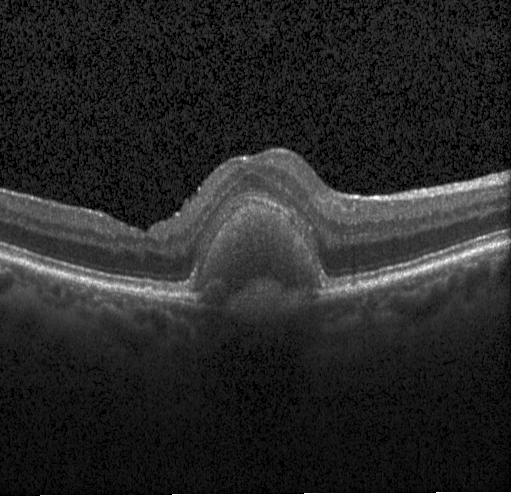 Retinal OCT B-scan. Fovea-centered. Spectral-domain OCT. Instrument: Heidelberg Spectralis — Impression: a choroidal neovascular membrane.